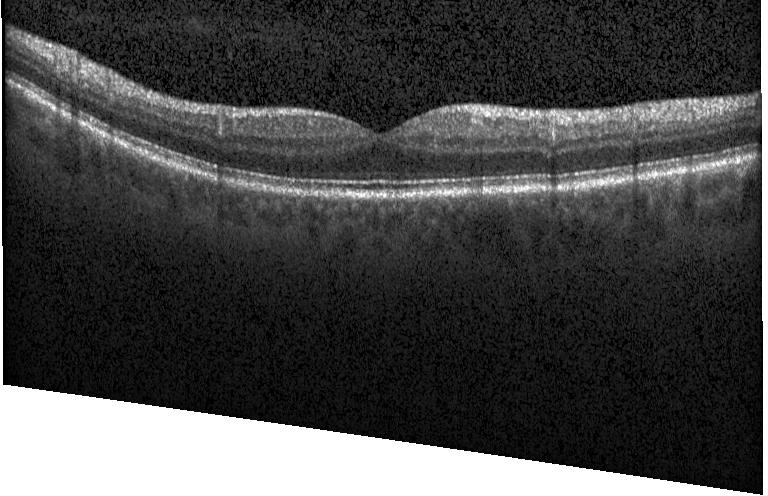

Finding: no CNV, no DME, and no drusen.